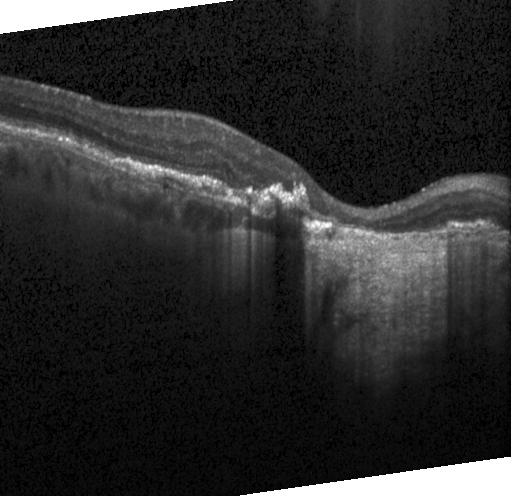

The scan shows a choroidal neovascular membrane.